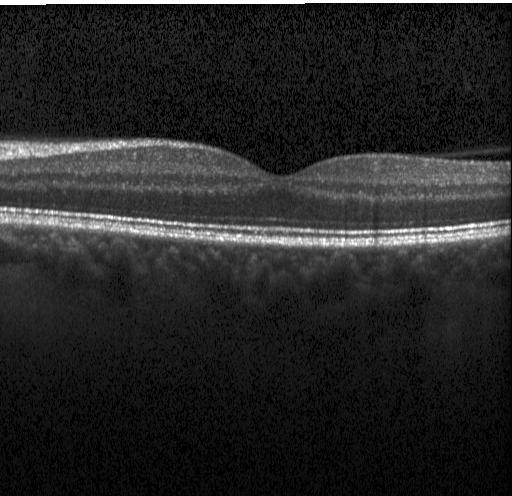 Spectral-domain OCT · optical coherence tomography B-scan · Heidelberg Spectralis
The scan shows neither choroidal neovascularization, diabetic macular edema, nor drusen.